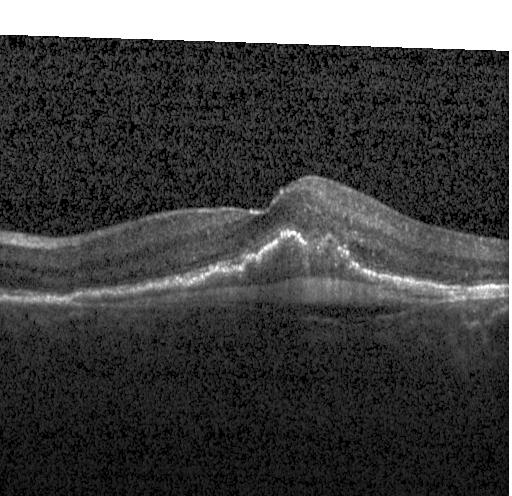
Retinal OCT cross-section, Heidelberg Spectralis OCT system, spectral-domain optical coherence tomography, fovea-centered. Finding: a choroidal neovascular membrane.